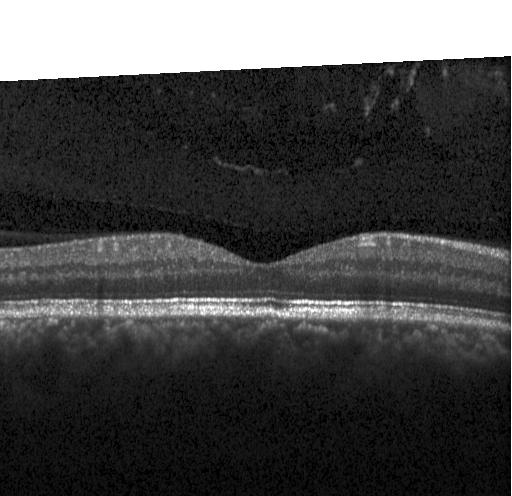 SD-OCT; acquired on a Heidelberg Spectralis; OCT line scan
Diagnosis: no evidence of choroidal neovascularization, diabetic macular edema, or drusen.